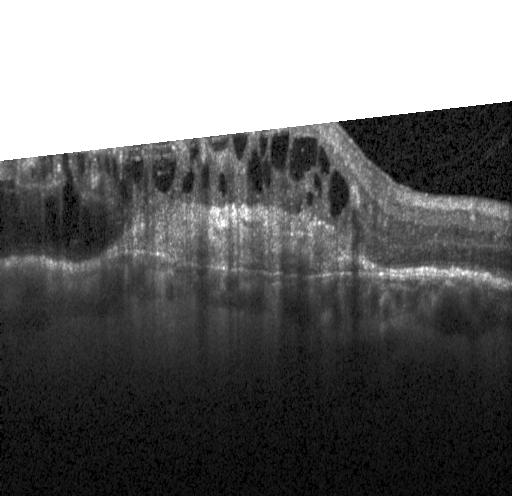 OCT B-scan — Impression: a choroidal neovascular membrane.